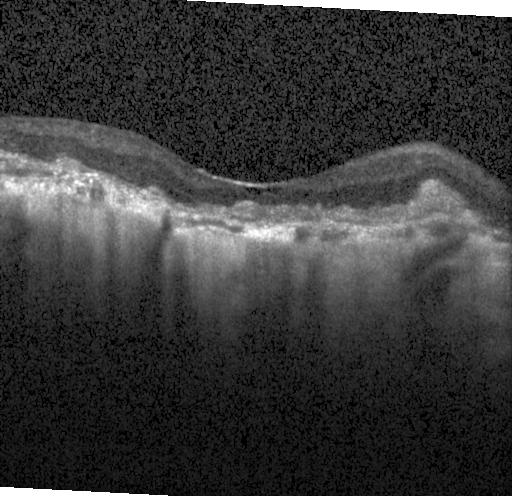
Optical coherence tomography scan.
The scan shows choroidal neovascularization (CNV).